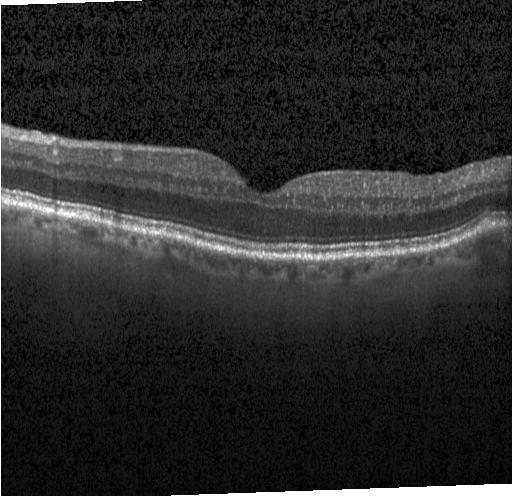

Retinal OCT B-scan.
Dx: no CNV, DME, or drusen.